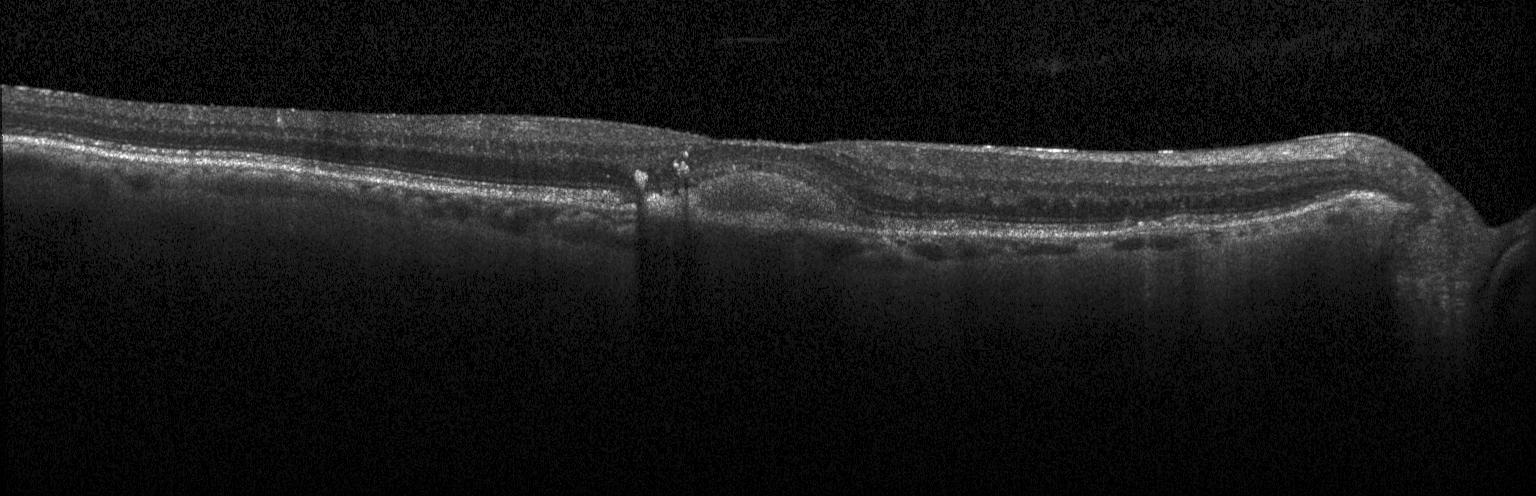

This B-scan demonstrates choroidal neovascularization (CNV).